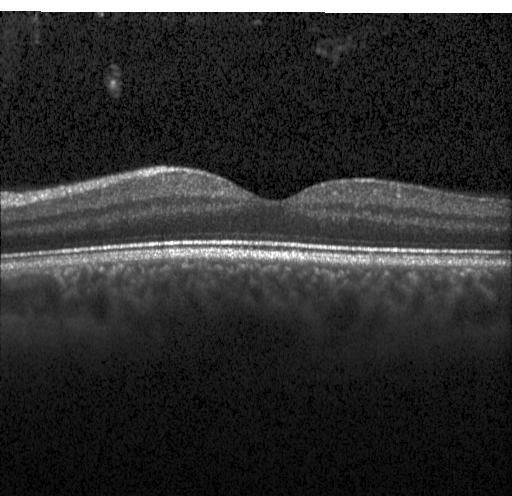

Spectral-domain OCT B-scan: neither CNV, DME, nor drusen.